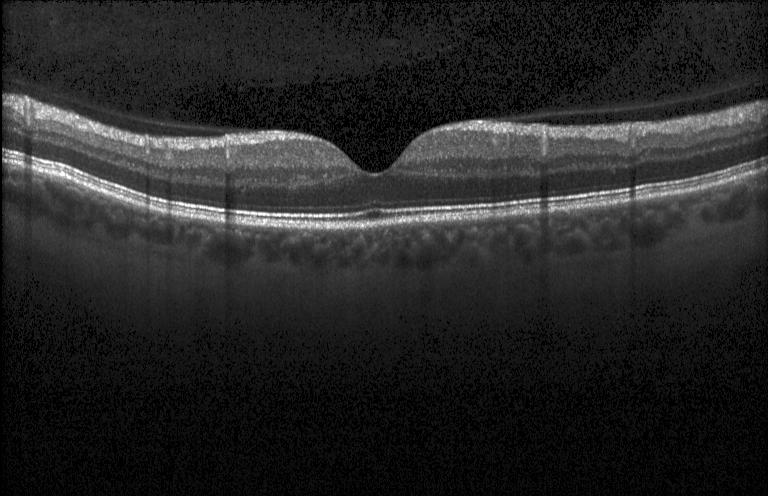 Macular OCT: neither choroidal neovascularization, diabetic macular edema, nor drusen.